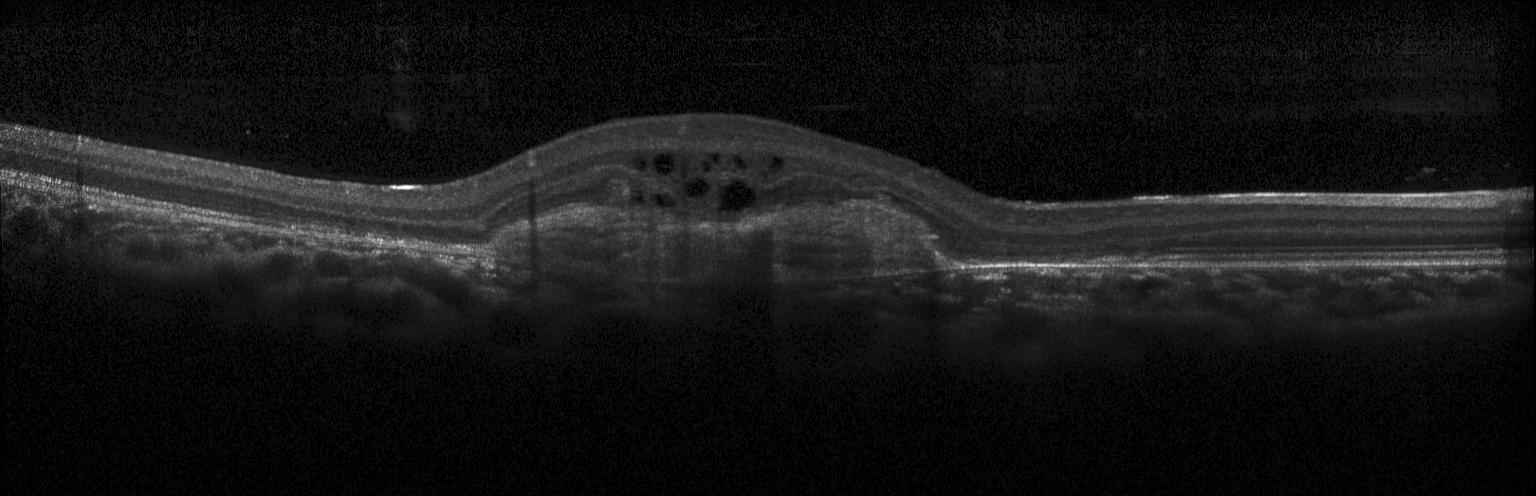

Heidelberg Spectralis. Retinal OCT B-scan. Spectral-domain optical coherence tomography
Macular OCT: a choroidal neovascular membrane.